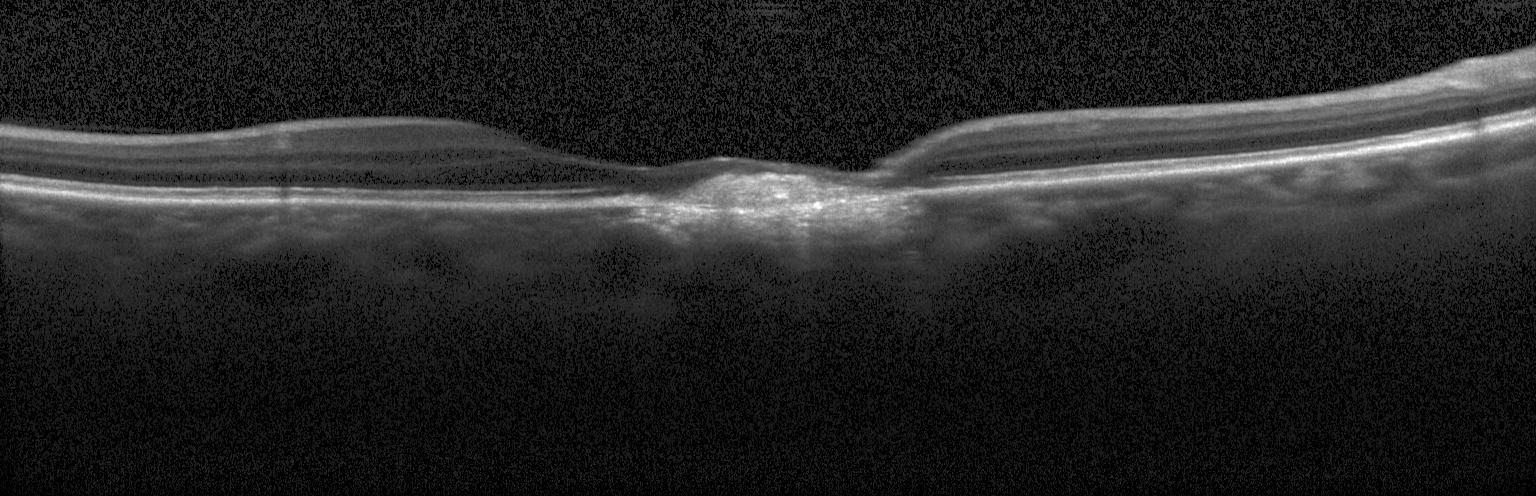
OCT line scan — The scan shows a choroidal neovascular membrane.